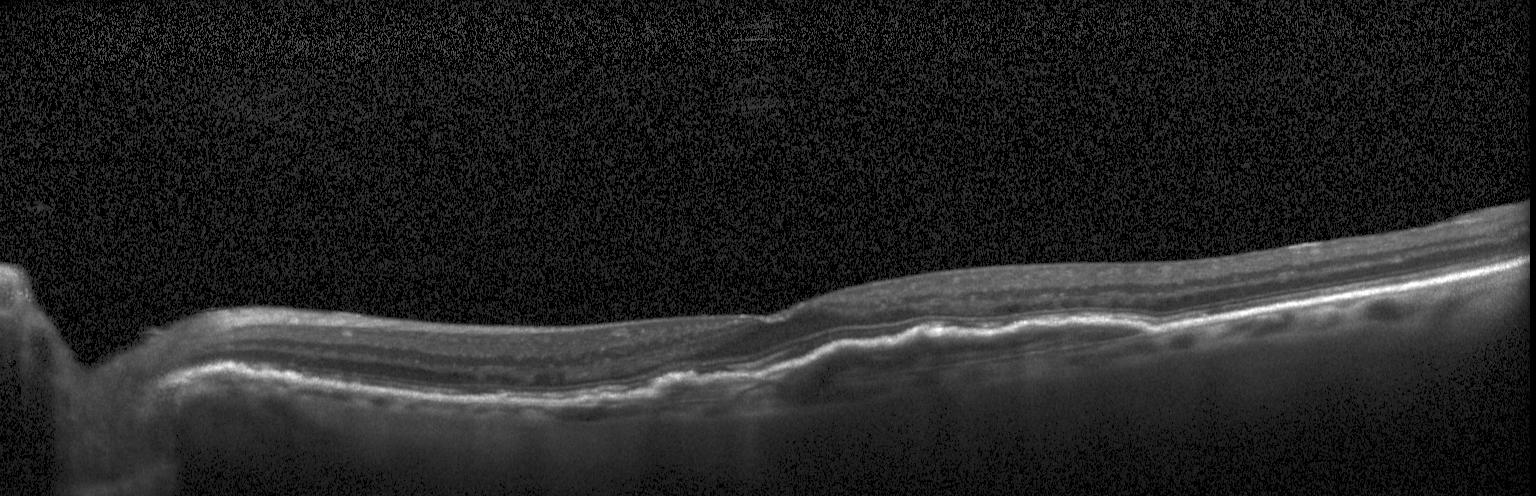 Heidelberg Spectralis OCT system. SD-OCT. OCT line scan
Dx: a choroidal neovascular membrane.